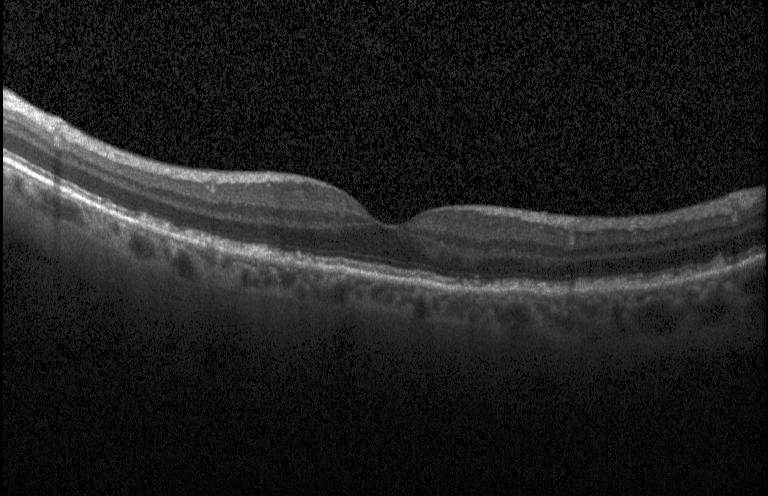

OCT scan showing sub-RPE drusenoid deposits.